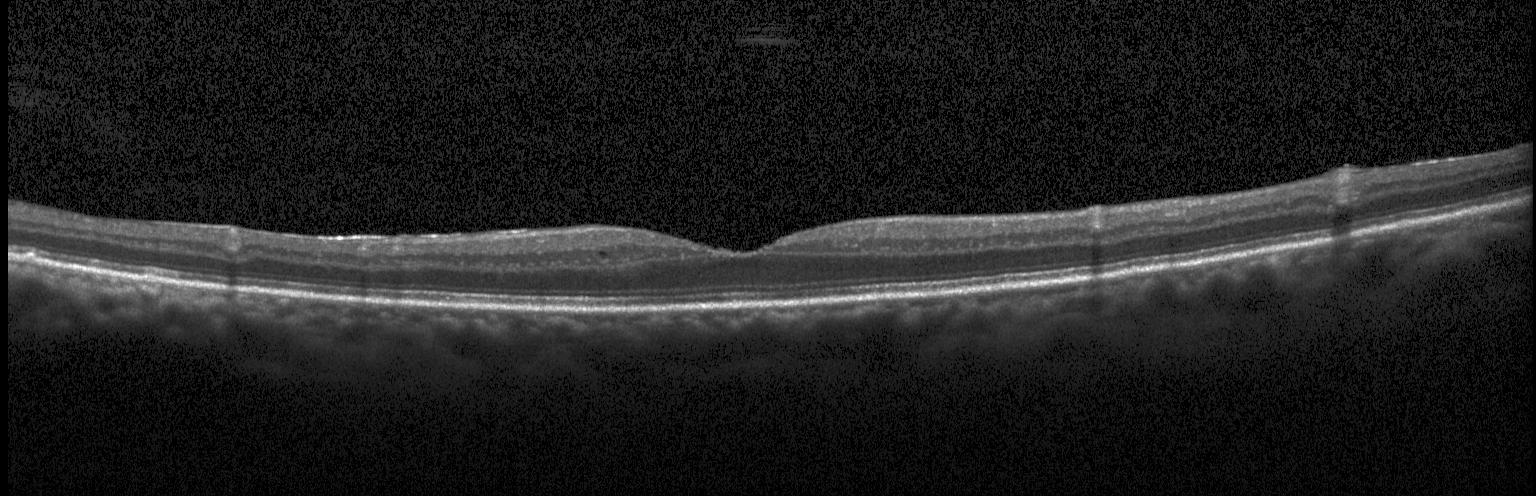 Macular OCT: no evidence of CNV, DME, or drusen.